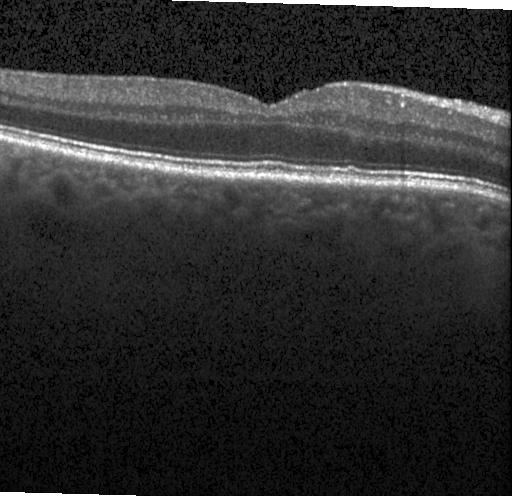
The scan shows no evidence of choroidal neovascularization, diabetic macular edema, or drusen.